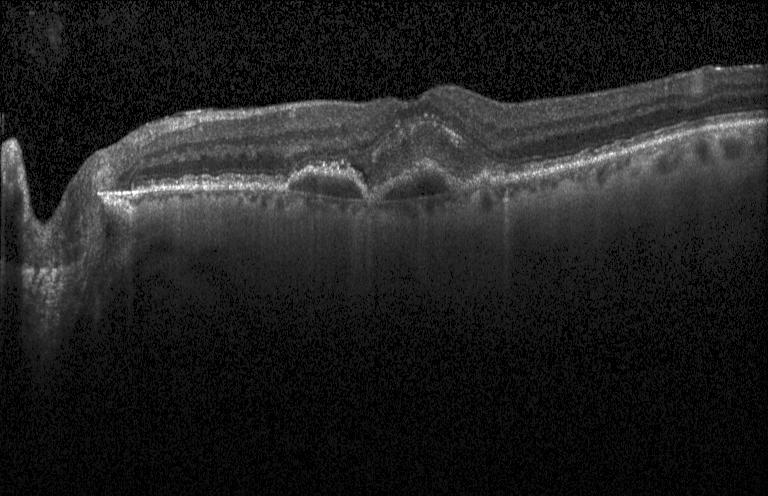
OCT B-scan showing choroidal neovascularization.